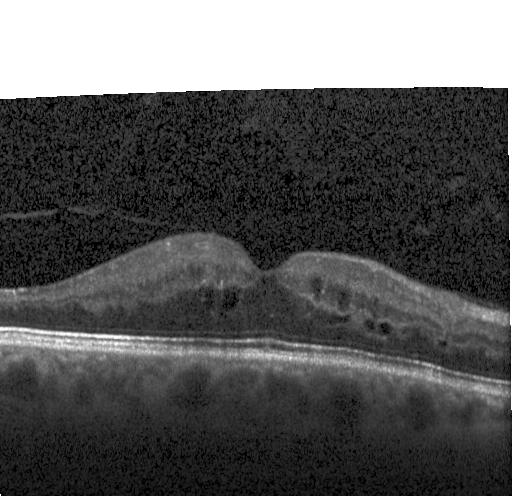 Finding: diabetic macular edema (DME).